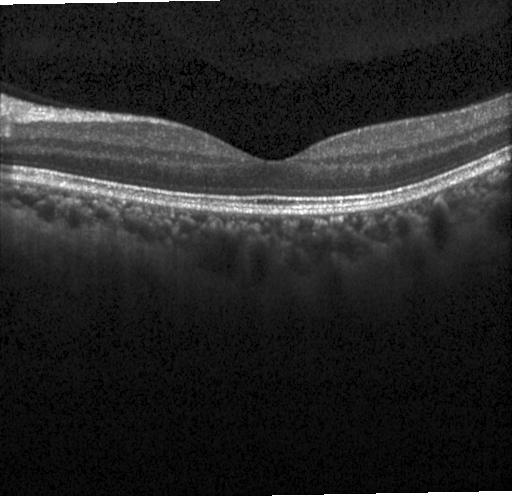

Heidelberg Spectralis · OCT line scan.
Dx: no CNV, no DME, and no drusen.